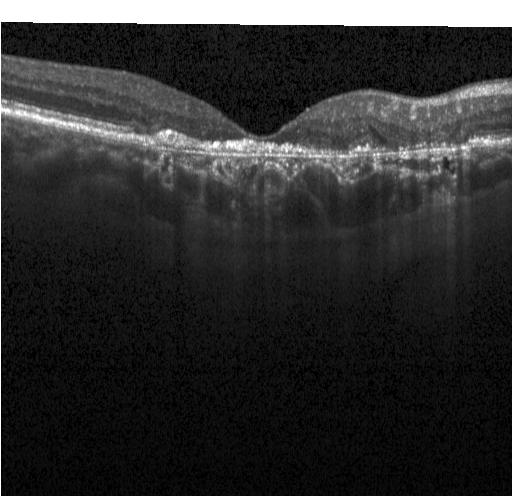 Optical coherence tomography scan, SD-OCT — A choroidal neovascular membrane.